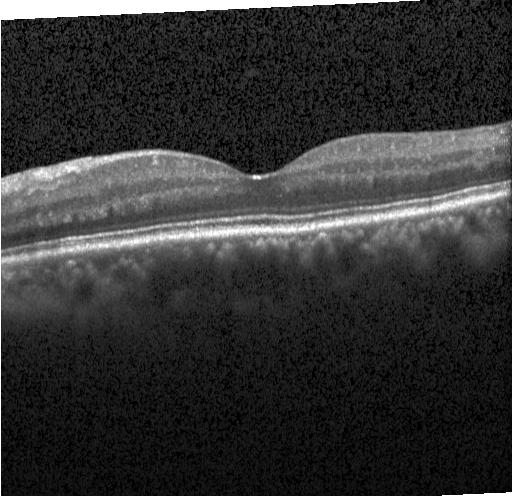

Spectral-domain OCT B-scan: no choroidal neovascularization, no diabetic macular edema, and no drusen.